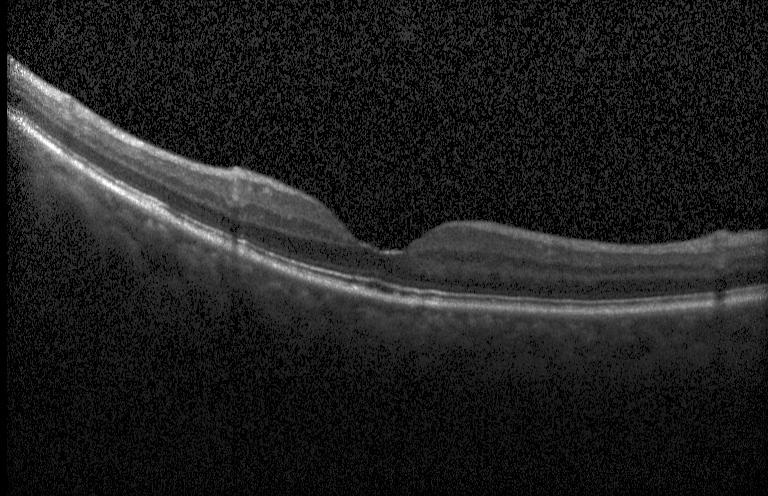
The scan shows no choroidal neovascularization, no diabetic macular edema, and no drusen.